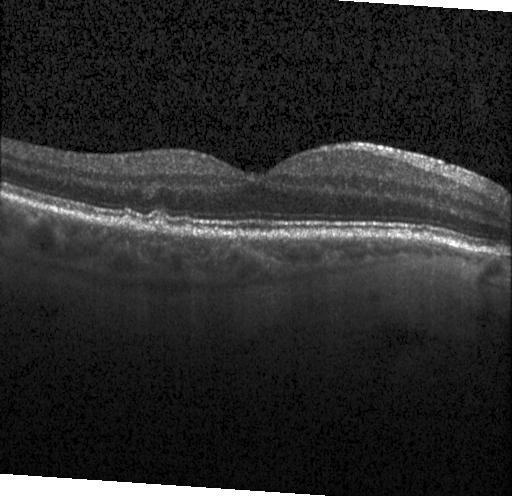

OCT scan showing drusen.